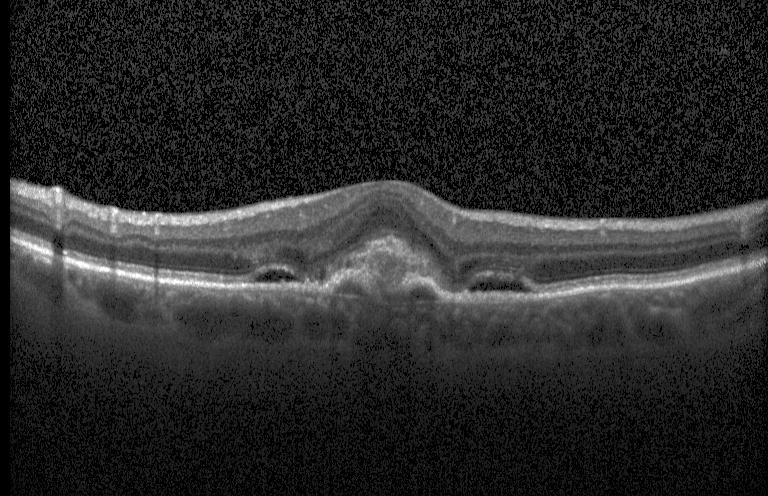
Spectral-domain optical coherence tomography, macular scan, optical coherence tomography B-scan.
The scan shows a choroidal neovascular membrane.